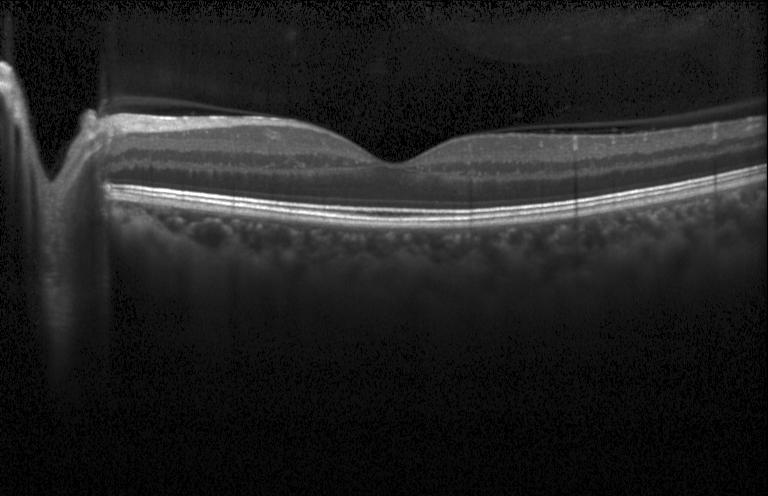 Heidelberg Spectralis OCT system. Fovea-centered. Optical coherence tomography B-scan. Dx: no evidence of CNV, DME, or drusen.